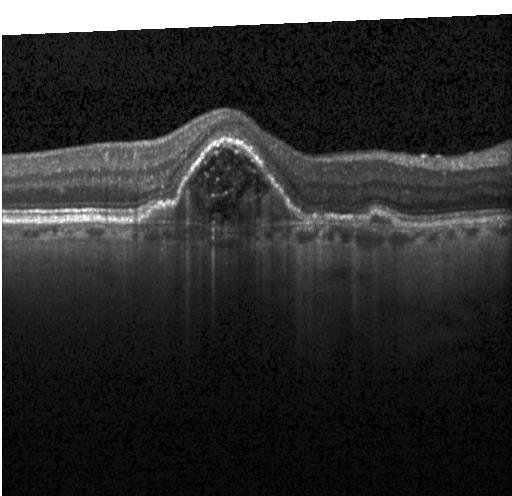

Finding: CNV.